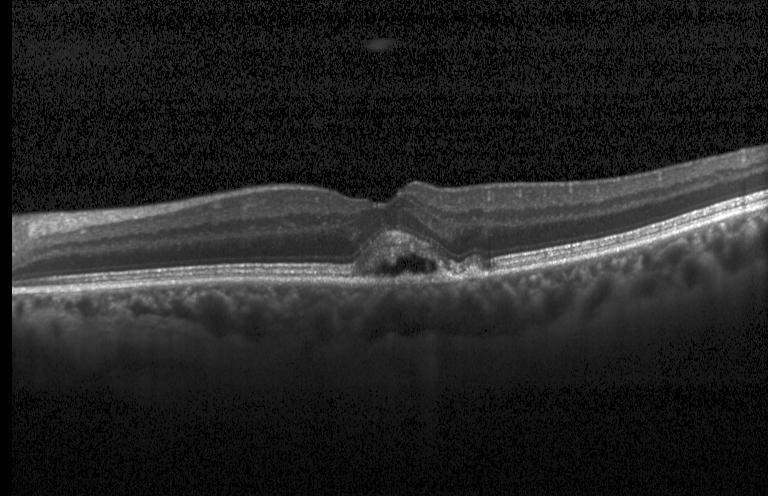
Dx: a choroidal neovascular membrane.